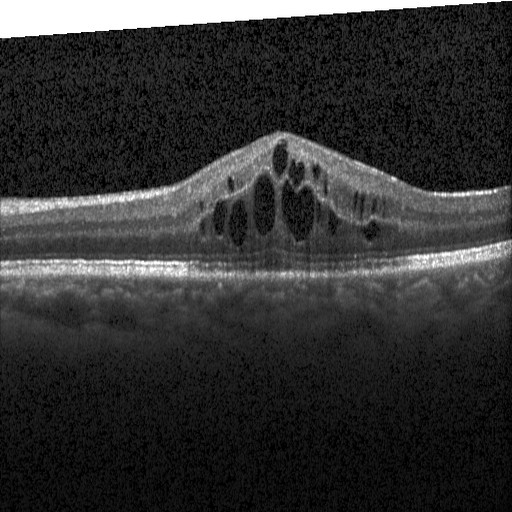

Retinal OCT cross-section — Diabetic macular edema (DME).